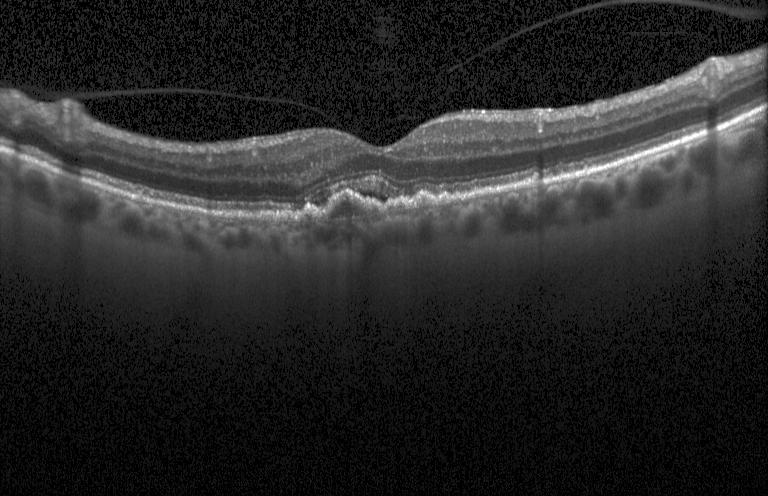

Optical coherence tomography B-scan.
Diagnosis: a choroidal neovascular membrane.